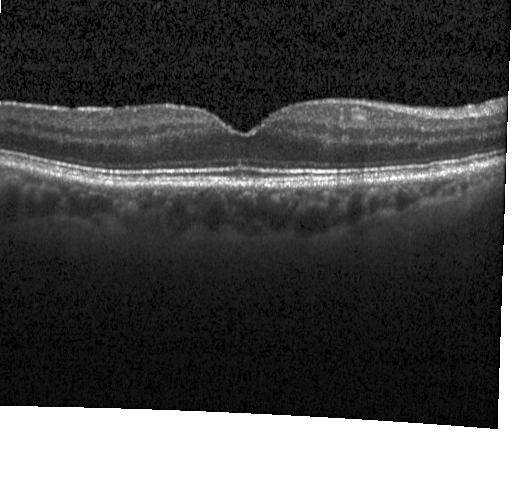 OCT scan showing no evidence of choroidal neovascularization, diabetic macular edema, or drusen.